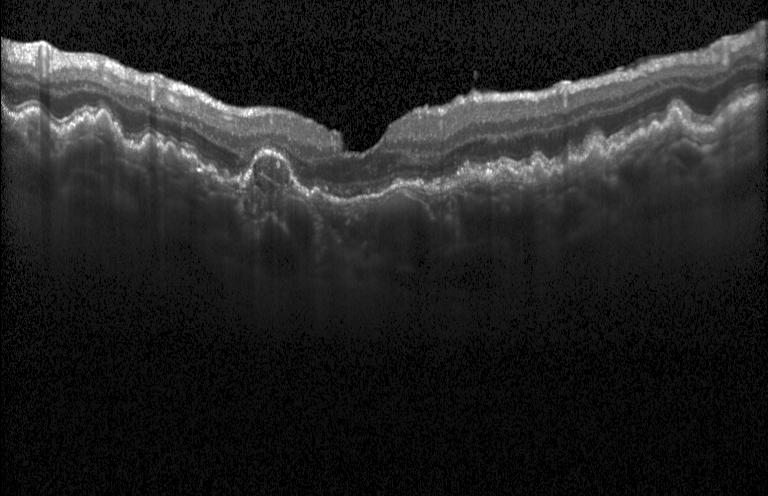 OCT B-scan showing a choroidal neovascular membrane.